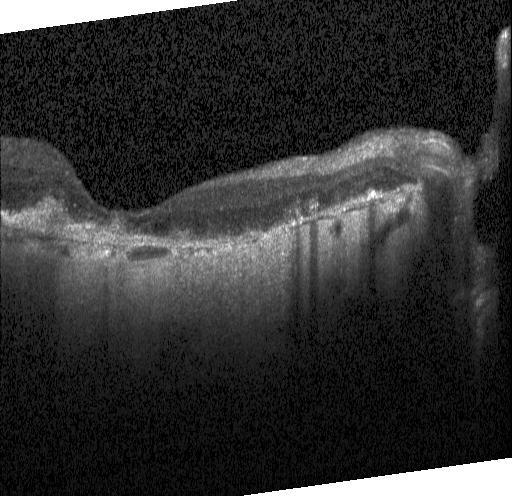 SD-OCT. Heidelberg Spectralis. Retinal OCT B-scan
Finding: CNV.